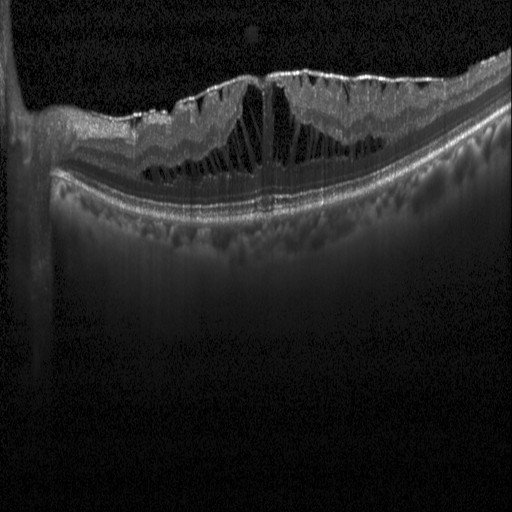 Finding: diabetic macular edema (DME).